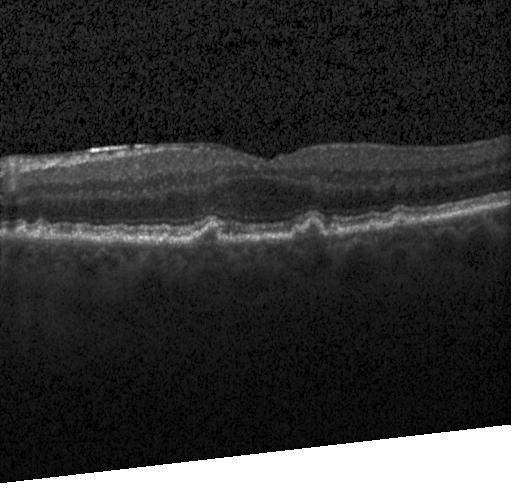
Optical coherence tomography B-scan. Through the macula. SD-OCT. Instrument: Heidelberg Spectralis
Assessment: multiple drusen.